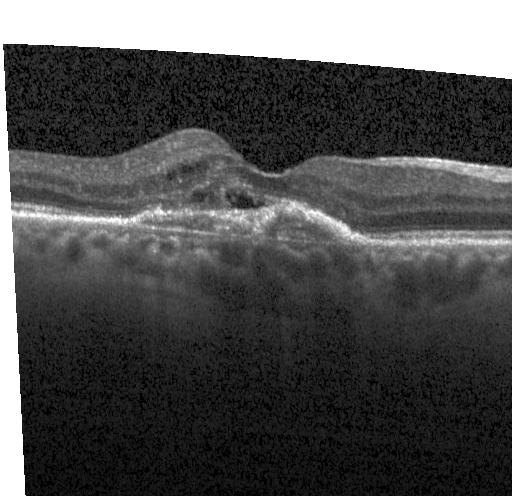
Macular scan. Instrument: Heidelberg Spectralis. Spectral-domain optical coherence tomography. Optical coherence tomography scan. Macular OCT: choroidal neovascularization.